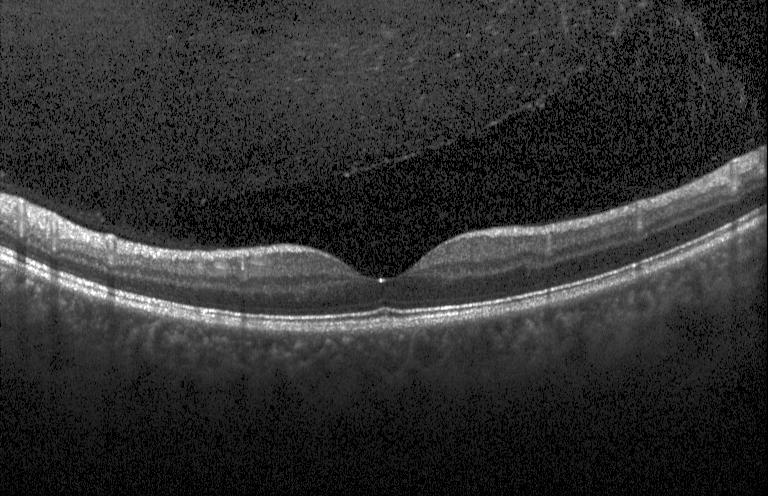
Centered on the fovea. Heidelberg Spectralis OCT system. OCT B-scan. Spectral-domain optical coherence tomography
Finding: no evidence of choroidal neovascularization, diabetic macular edema, or drusen.